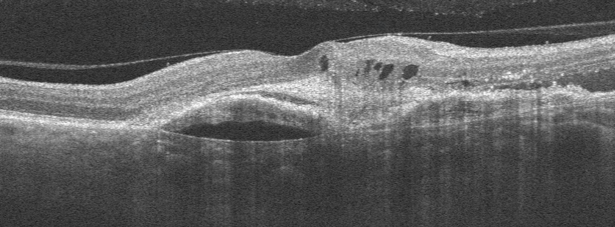

OCT finding: age-related macular degeneration.